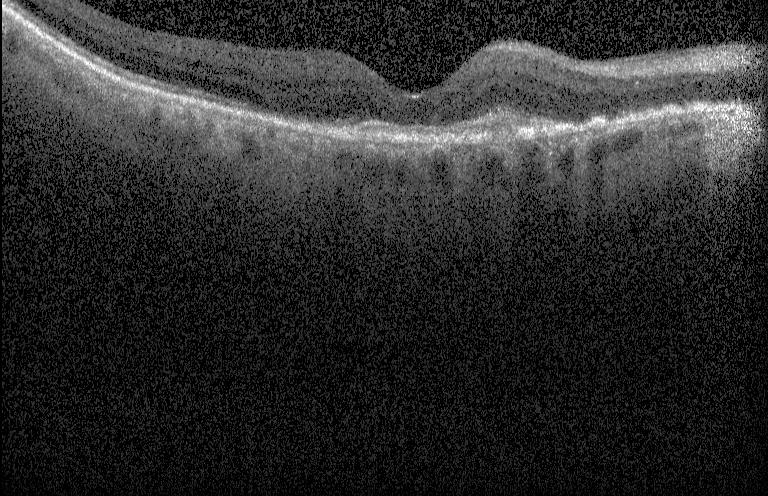
Spectral-domain optical coherence tomography · optical coherence tomography B-scan · instrument: Heidelberg Spectralis. Macular OCT: choroidal neovascularization.